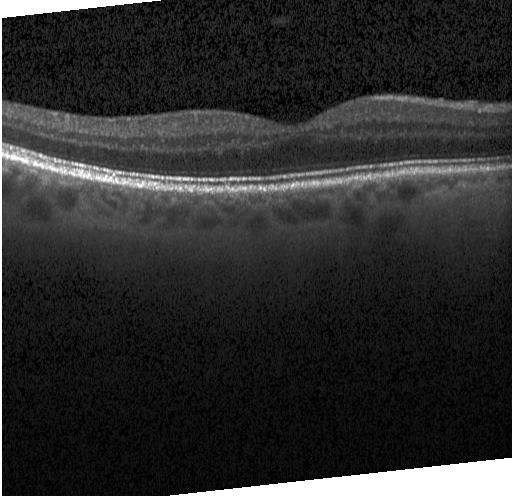 SD-OCT; instrument: Heidelberg Spectralis; optical coherence tomography B-scan; horizontal scan through the fovea. Finding: neither CNV, DME, nor drusen.